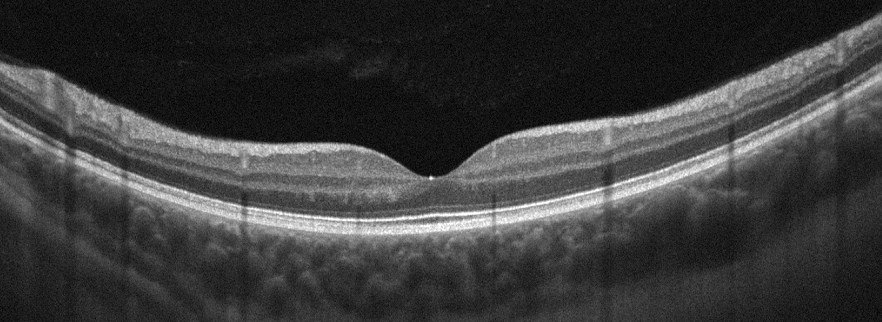 Optovue Avanti RTVue XR. Optical coherence tomography scan. Right eye. This B-scan demonstrates no evidence of AMD, DME, ERM, RAO, RVO, or VID.